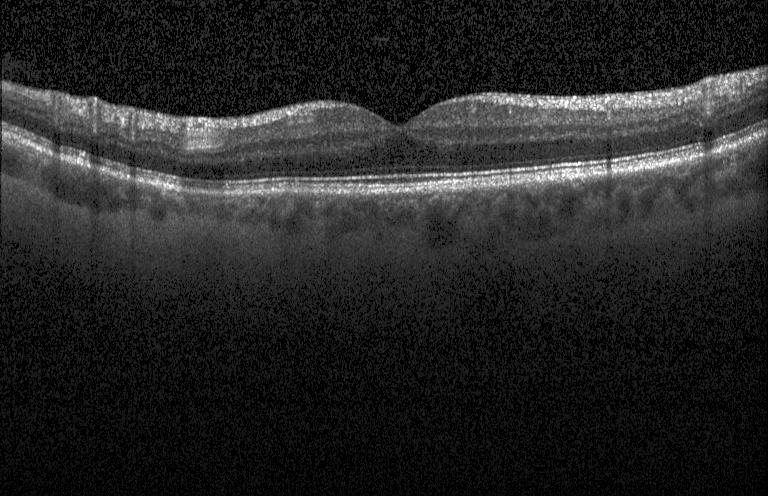 Diagnosis: no CNV, DME, or drusen.